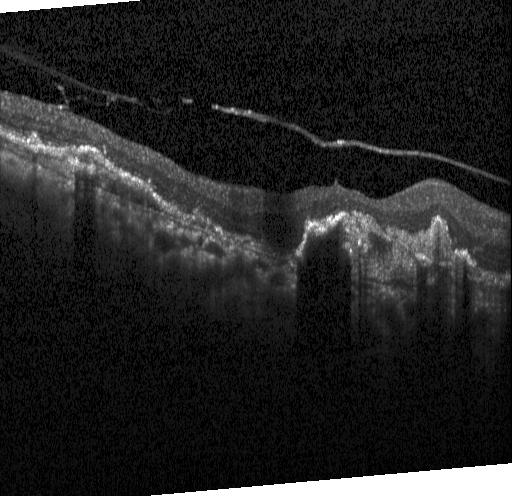

Finding: a choroidal neovascular membrane.